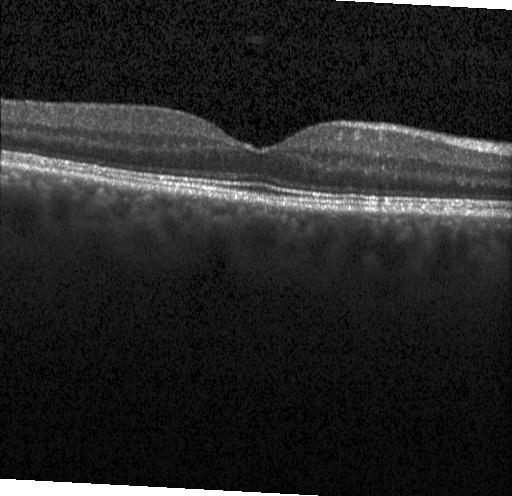 Dx: neither choroidal neovascularization, diabetic macular edema, nor drusen.